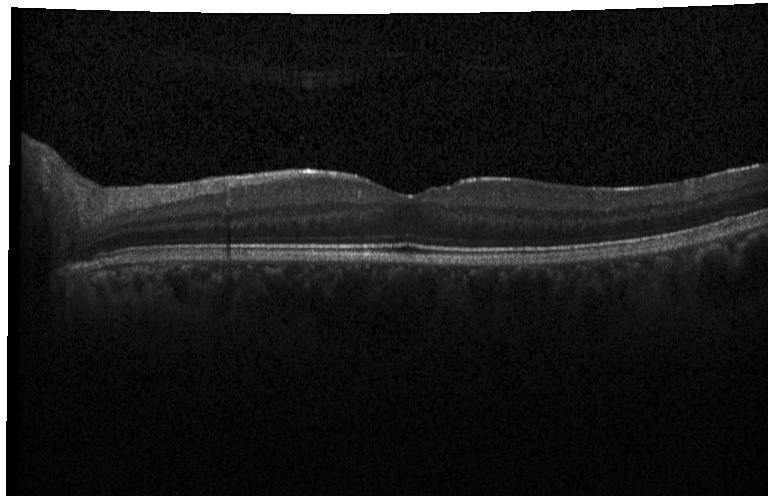
Impression: neither choroidal neovascularization, diabetic macular edema, nor drusen.